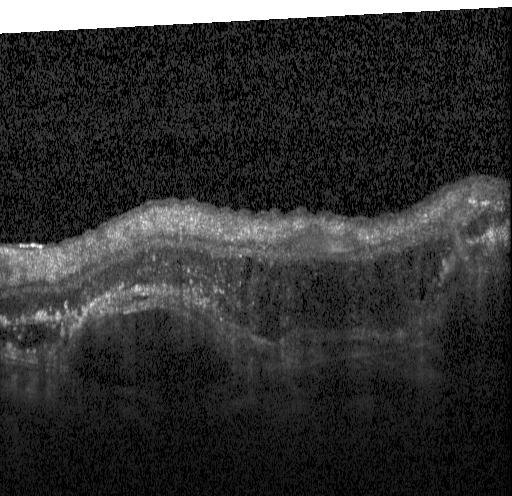 Diagnosis: a choroidal neovascular membrane.